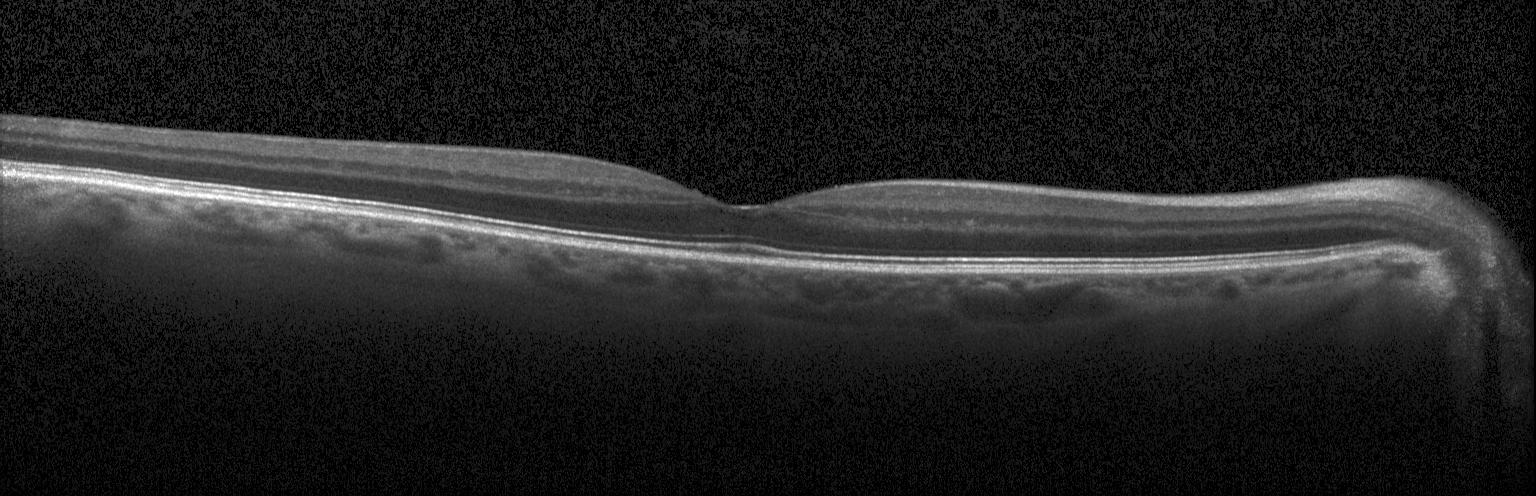

Horizontal scan through the fovea, SD-OCT, OCT B-scan
Dx: no evidence of choroidal neovascularization, diabetic macular edema, or drusen.